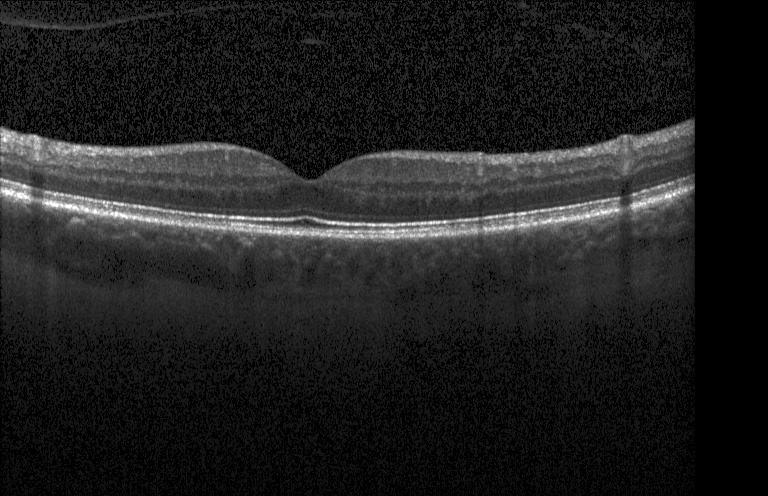
Optical coherence tomography scan. Spectral-domain optical coherence tomography. Fovea-centered.
No choroidal neovascularization, diabetic macular edema, or drusen.